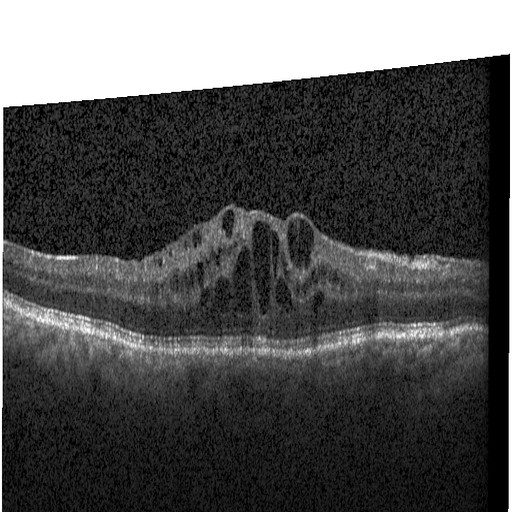
Dx: DME.